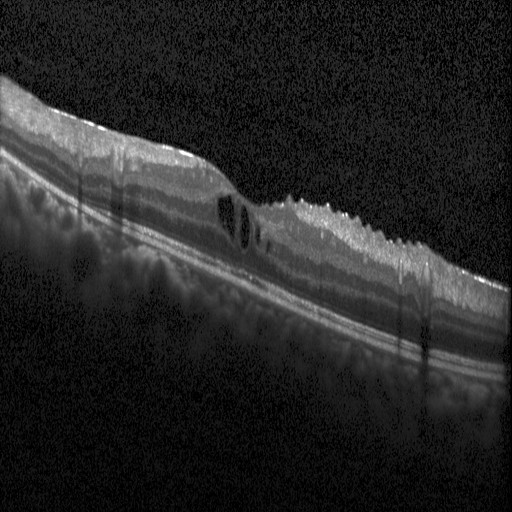 Spectral-domain optical coherence tomography. Retinal OCT B-scan. Heidelberg Spectralis. Centered on the fovea. Macular OCT: DME.